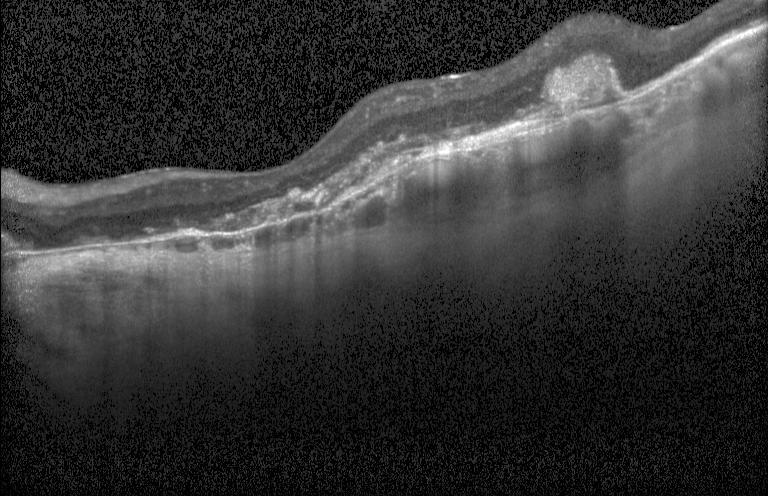 Spectral-domain OCT, OCT B-scan, Heidelberg Spectralis OCT system, through the macula — Assessment: choroidal neovascularization (CNV).